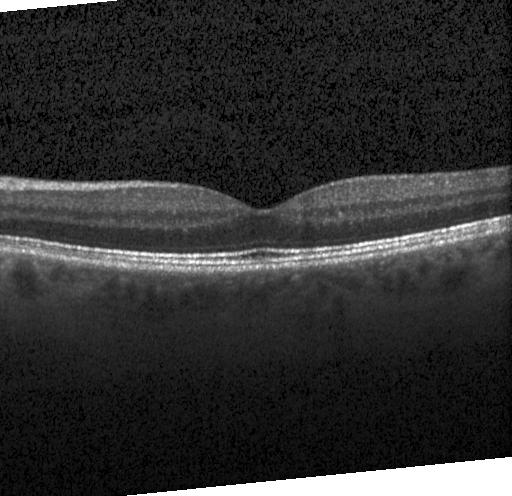
Optical coherence tomography scan, spectral-domain OCT — No choroidal neovascularization, diabetic macular edema, or drusen.